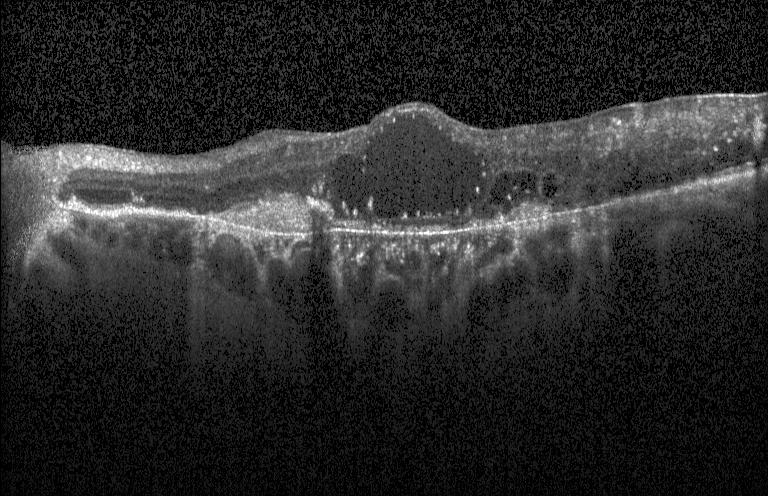 Optical coherence tomography scan, SD-OCT
Finding: a choroidal neovascular membrane.